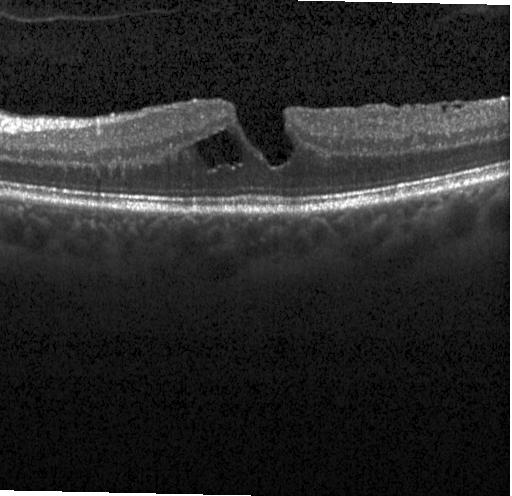

Macular OCT: diabetic macular edema (DME).